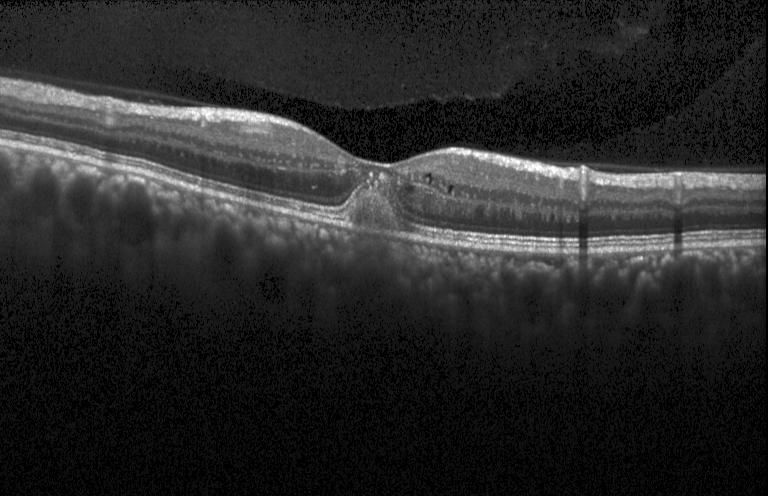
Retinal OCT cross-section showing CNV.